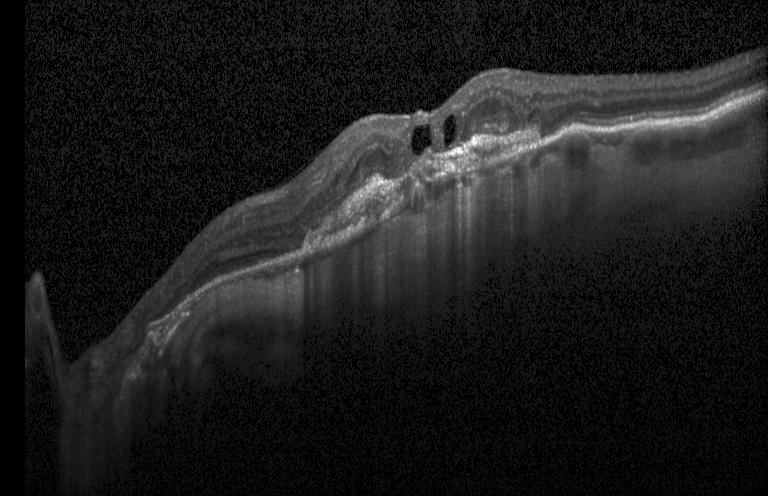

OCT scan showing a choroidal neovascular membrane.